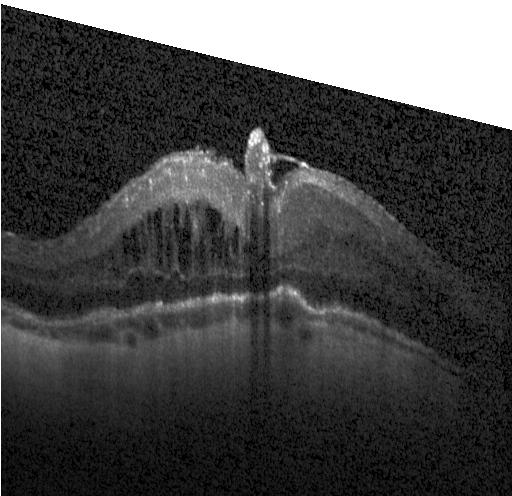
Retinal OCT cross-section showing diabetic macular edema.